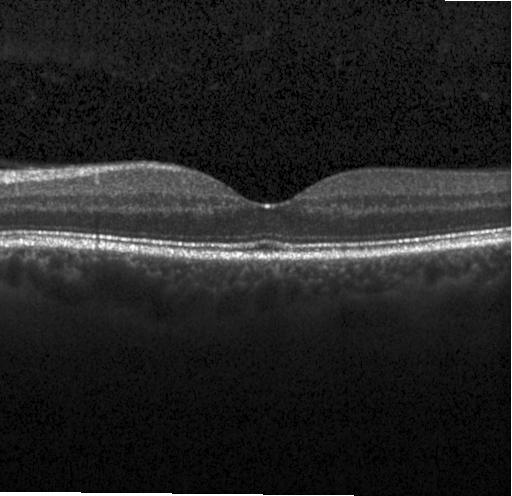

Macular scan. OCT line scan. Spectral-domain OCT. Impression: neither choroidal neovascularization, diabetic macular edema, nor drusen.